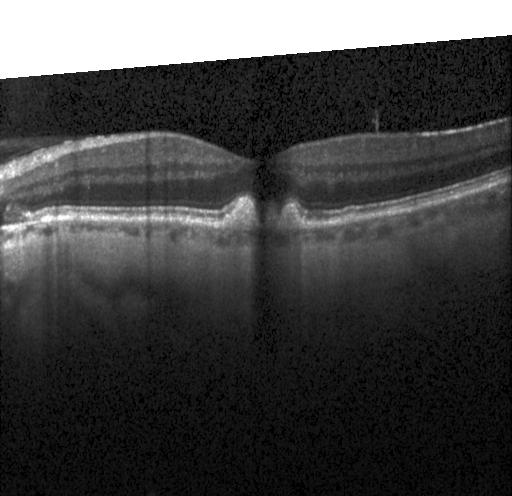
Spectral-domain OCT B-scan: sub-RPE drusenoid deposits.